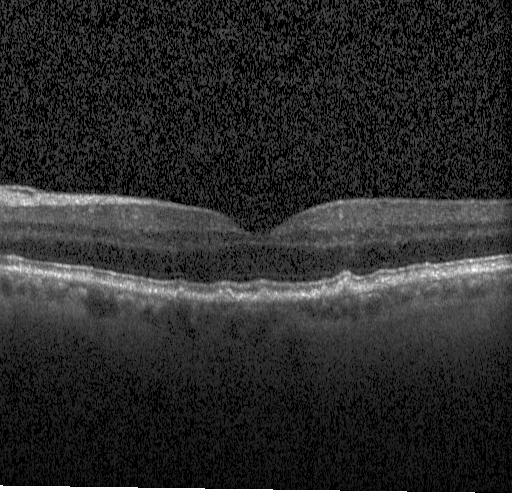
Finding: multiple drusen.